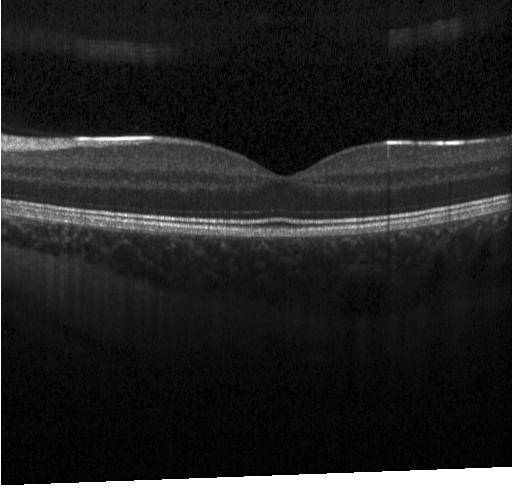 Spectral-domain OCT B-scan: neither choroidal neovascularization, diabetic macular edema, nor drusen.